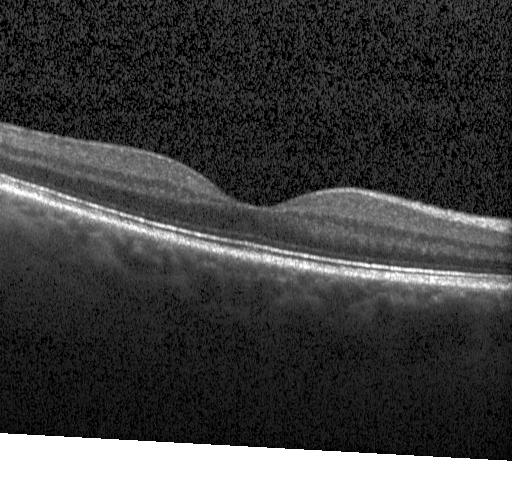

Spectral-domain OCT, fovea-centered, retinal OCT B-scan.
Diagnosis: no CNV, no DME, and no drusen.